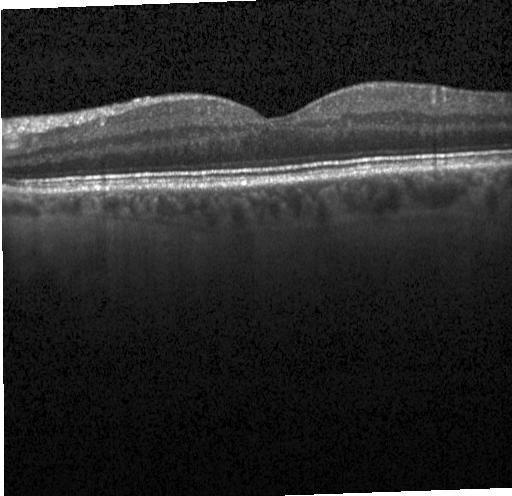

Acquired on a Heidelberg Spectralis; OCT line scan — OCT finding: neither choroidal neovascularization, diabetic macular edema, nor drusen.